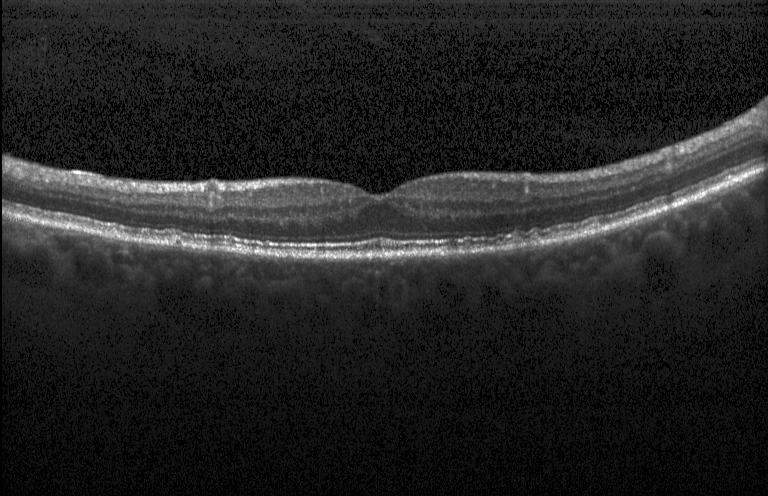 Impression: sub-RPE drusenoid deposits.